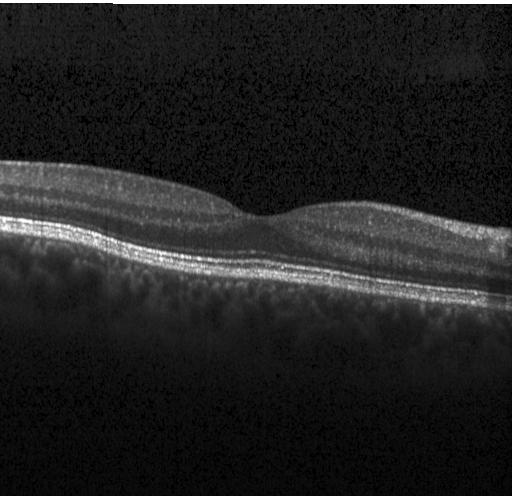
Optical coherence tomography scan, spectral-domain OCT — This B-scan demonstrates neither CNV, DME, nor drusen.